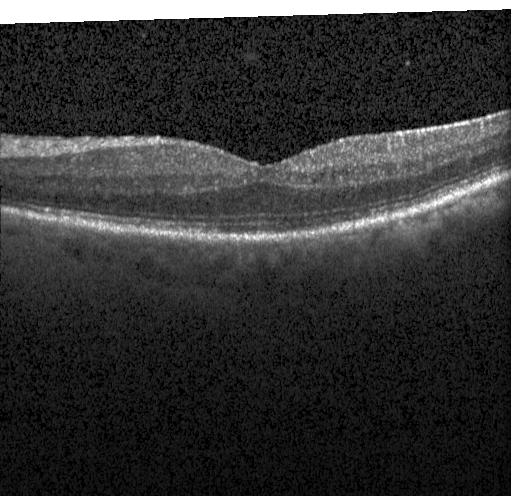 Optical coherence tomography B-scan
No CNV, DME, or drusen.